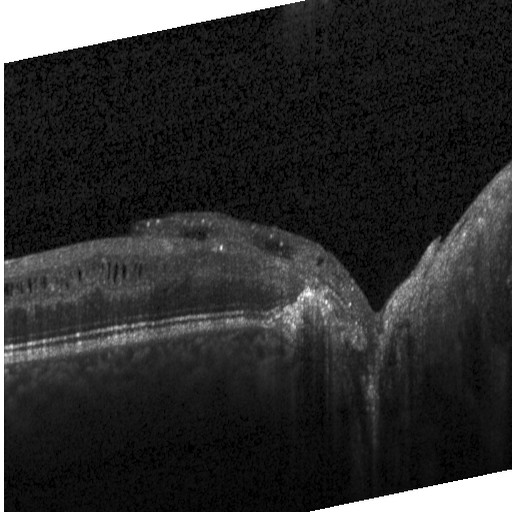 Heidelberg Spectralis, retinal OCT B-scan — This B-scan demonstrates diabetic macular edema.